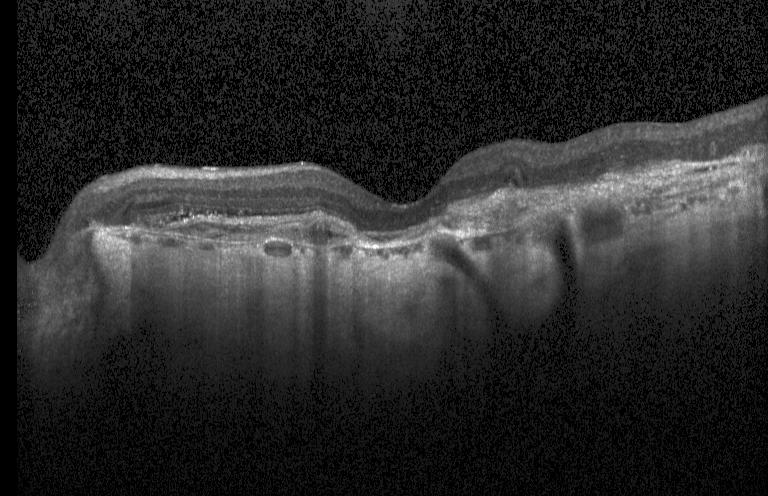
Retinal OCT B-scan; centered on the fovea; spectral-domain optical coherence tomography. CNV.